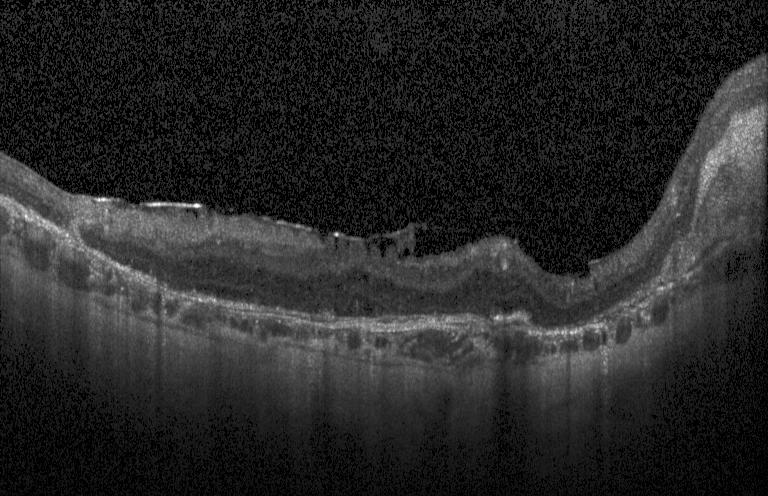
OCT line scan. OCT finding: a choroidal neovascular membrane.